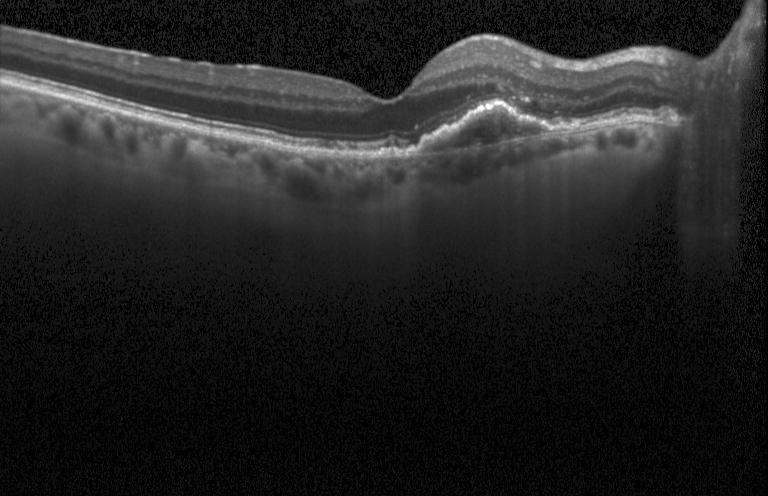 Optical coherence tomography B-scan · Heidelberg Spectralis OCT system.
The scan shows a choroidal neovascular membrane.